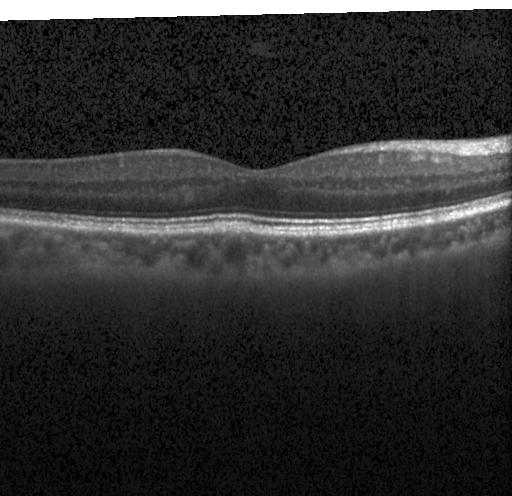 The scan shows neither CNV, DME, nor drusen.